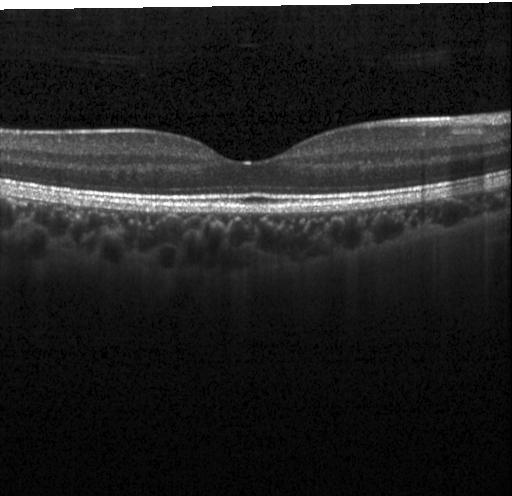
Diagnosis: neither CNV, DME, nor drusen.